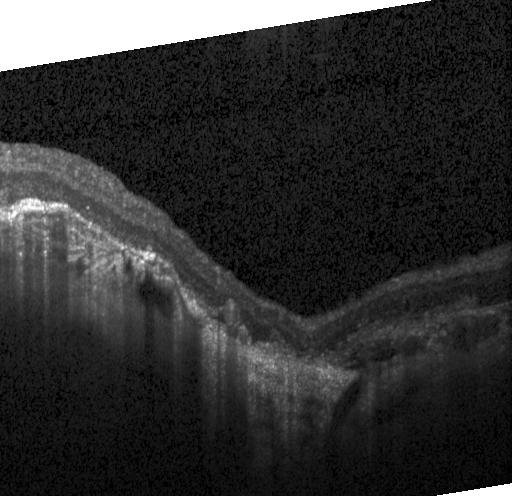
Spectral-domain OCT B-scan: a choroidal neovascular membrane.